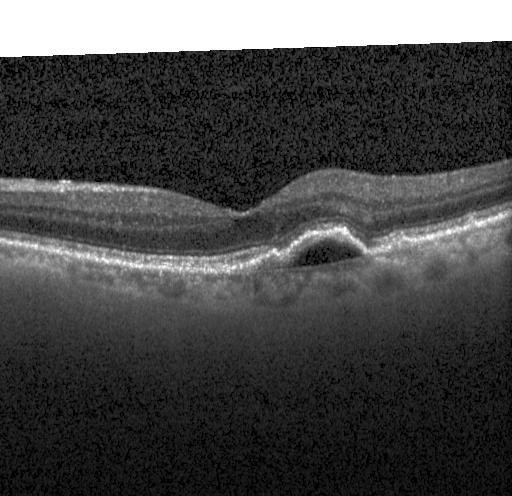
OCT B-scan showing a choroidal neovascular membrane.